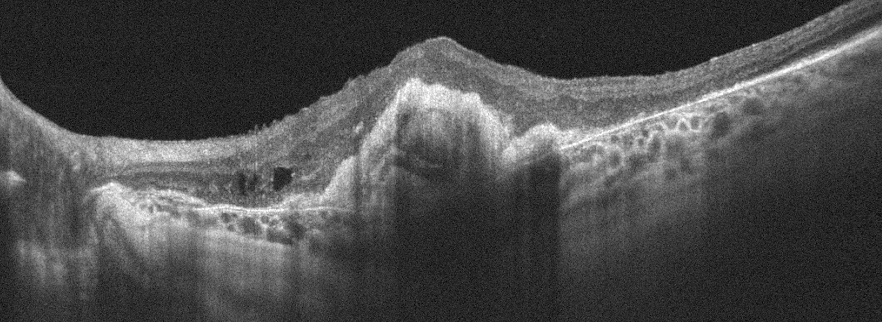

OS, macular scan, retinal OCT cross-section.
Finding: age-related macular degeneration (AMD).